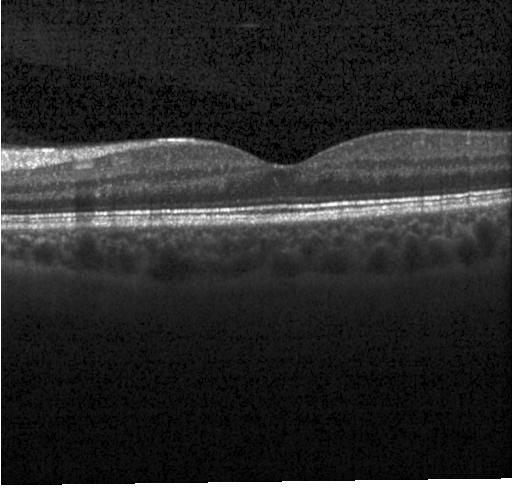 Retinal OCT cross-section. Macular OCT: neither choroidal neovascularization, diabetic macular edema, nor drusen.